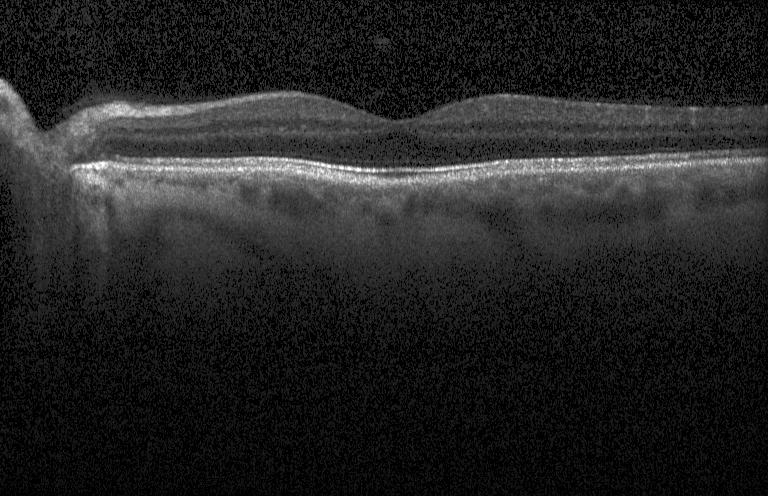 Horizontal scan through the fovea · spectral-domain OCT · OCT line scan — The scan shows neither choroidal neovascularization, diabetic macular edema, nor drusen.